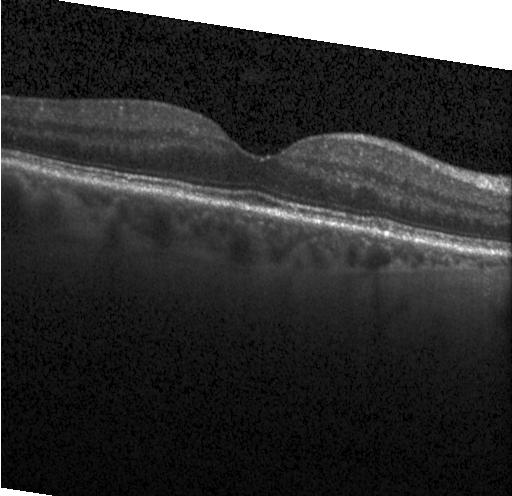

Diagnosis: no choroidal neovascularization, diabetic macular edema, or drusen.